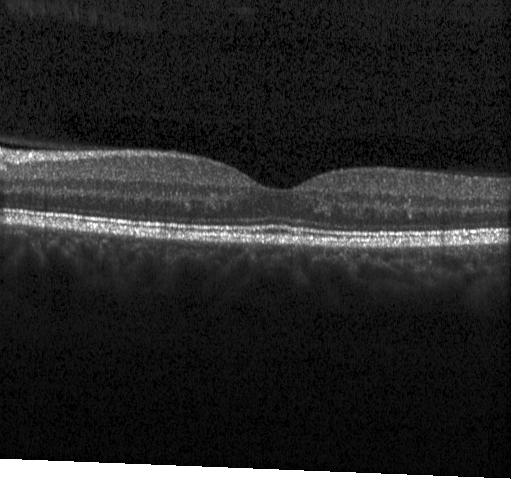

Retinal OCT cross-section; spectral-domain OCT — Impression: neither choroidal neovascularization, diabetic macular edema, nor drusen.